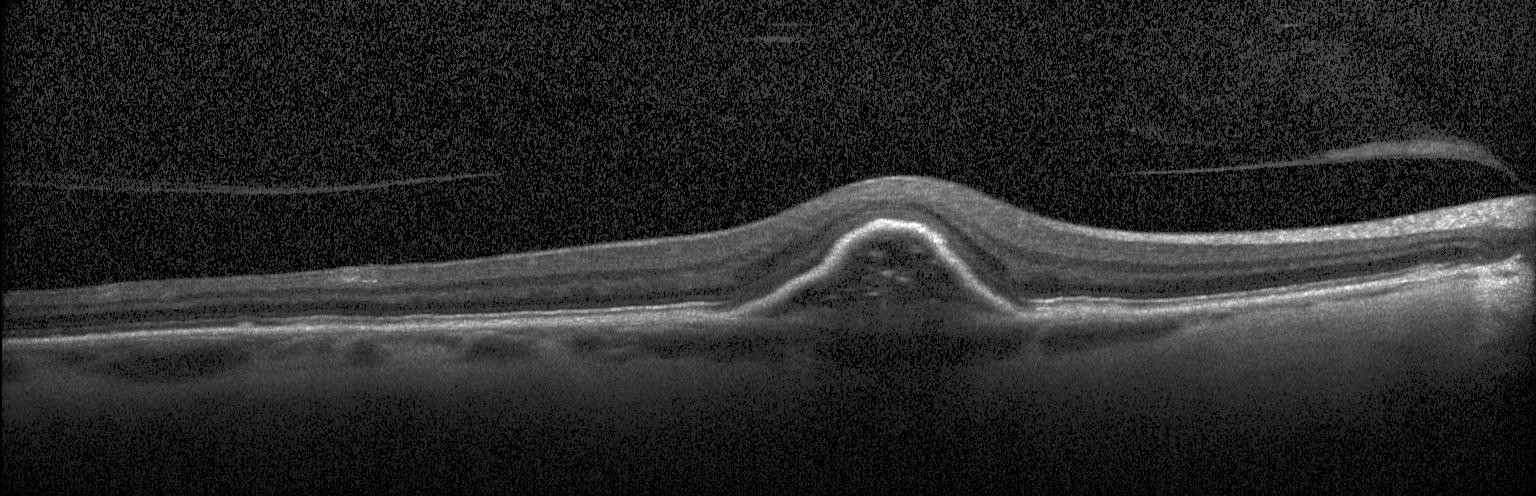

Dx: choroidal neovascularization.